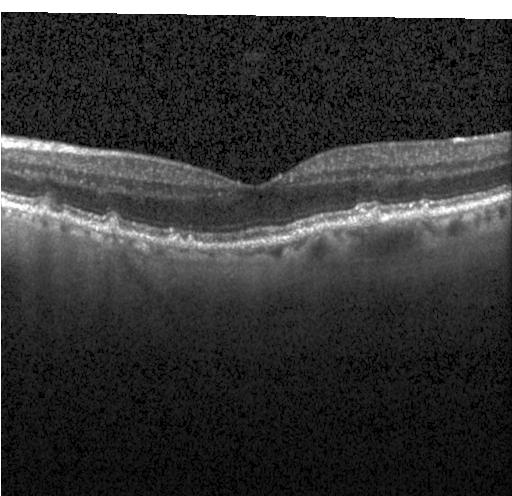 Optical coherence tomography scan — Diagnosis: sub-RPE drusenoid deposits.